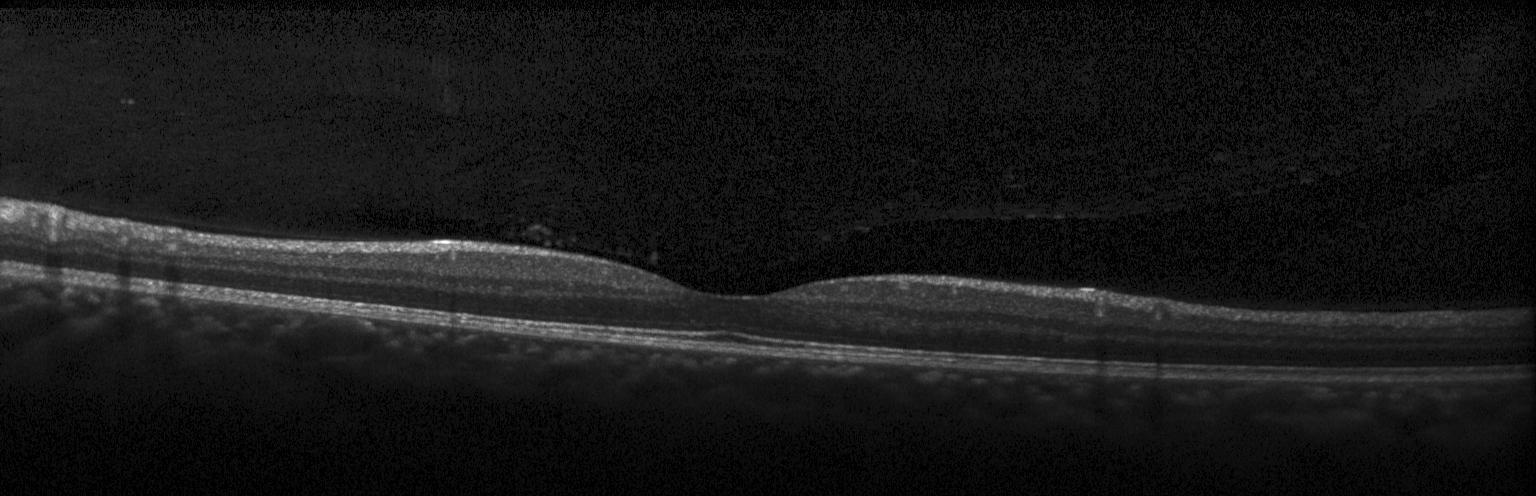 Optical coherence tomography scan
Impression: neither choroidal neovascularization, diabetic macular edema, nor drusen.